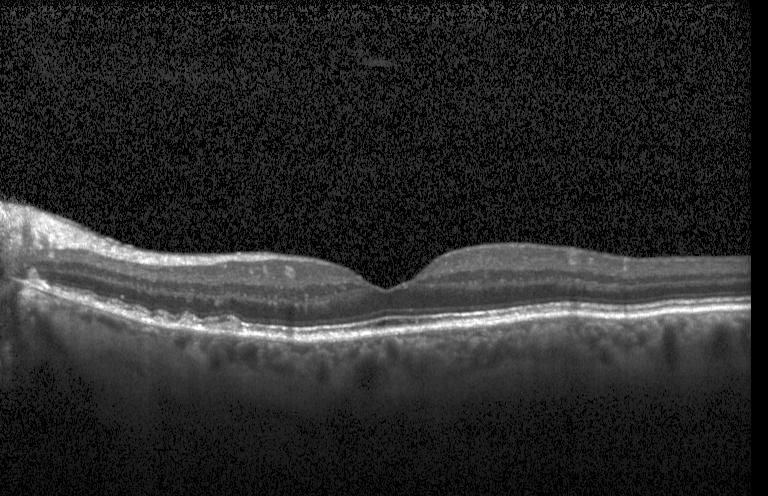
Macular scan; spectral-domain optical coherence tomography; acquired on a Heidelberg Spectralis; OCT B-scan. Dx: sub-RPE drusenoid deposits.